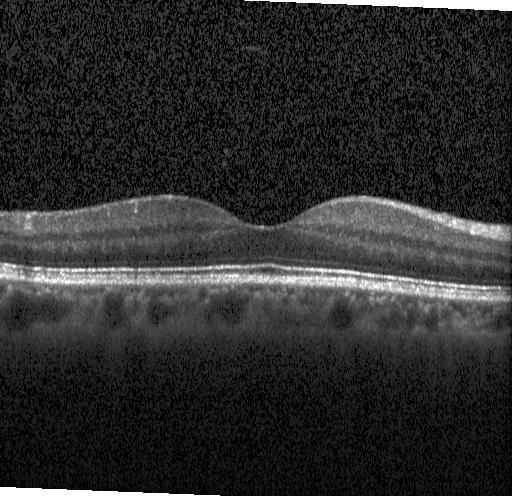

Spectral-domain optical coherence tomography, optical coherence tomography B-scan
The scan shows neither choroidal neovascularization, diabetic macular edema, nor drusen.